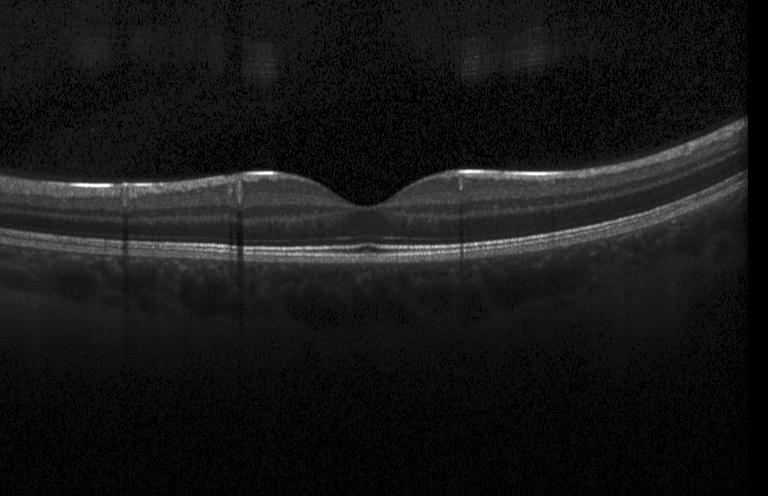

Spectral-domain OCT B-scan: no evidence of choroidal neovascularization, diabetic macular edema, or drusen.